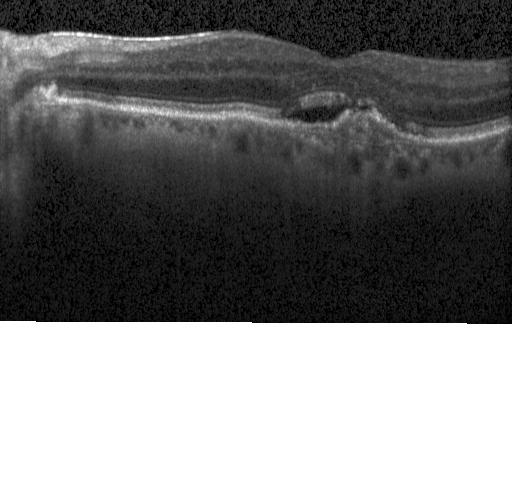
Macular OCT demonstrating a choroidal neovascular membrane.